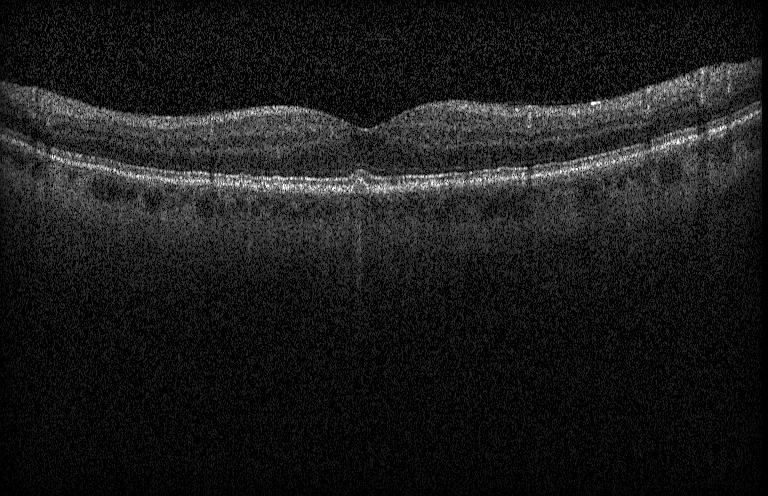 The scan shows sub-RPE drusenoid deposits.